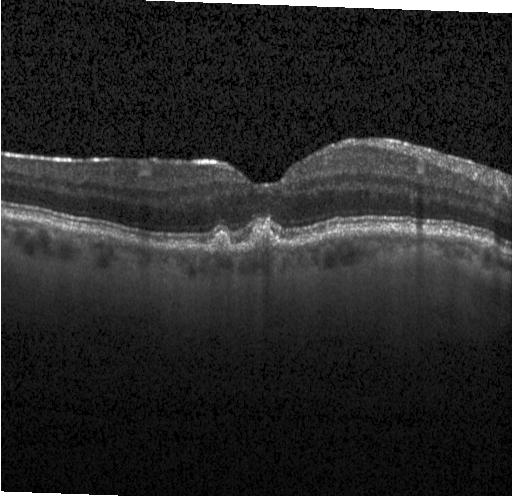 Acquired on a Heidelberg Spectralis, OCT B-scan, spectral-domain OCT.
Diagnosis: sub-RPE drusenoid deposits.